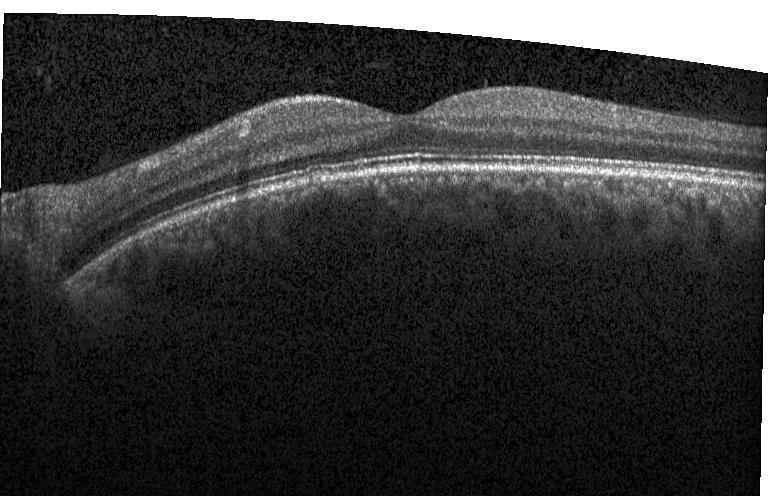

Acquired on a Heidelberg Spectralis · SD-OCT · retinal OCT cross-section.
Diagnosis: neither choroidal neovascularization, diabetic macular edema, nor drusen.